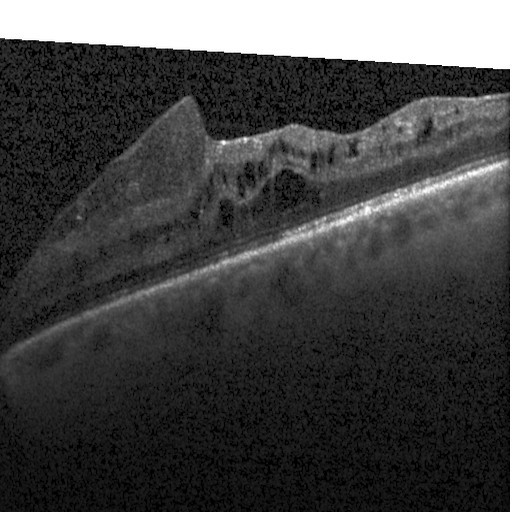
SD-OCT · macular scan · Heidelberg Spectralis OCT system · OCT line scan
Impression: DME.